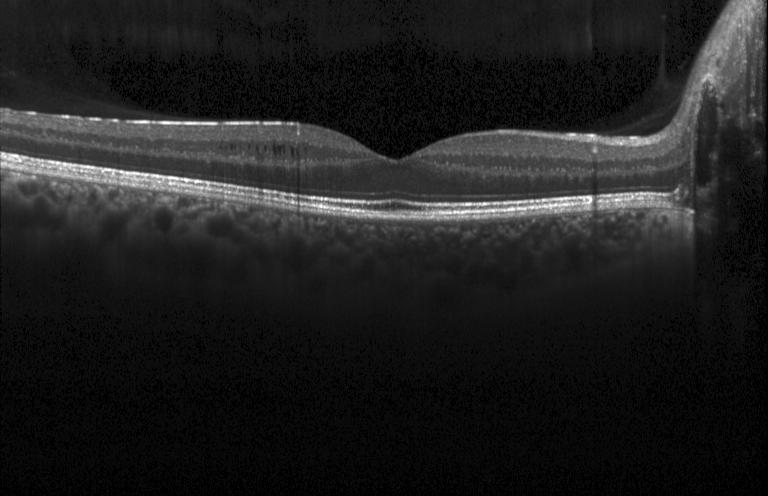 Retinal OCT cross-section
OCT finding: no evidence of choroidal neovascularization, diabetic macular edema, or drusen.